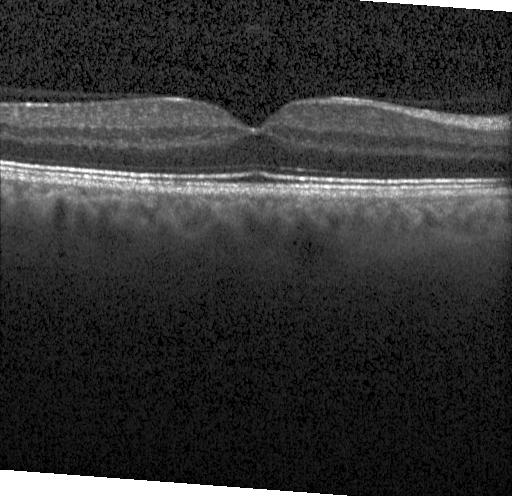

OCT line scan · spectral-domain OCT
This B-scan demonstrates no choroidal neovascularization, no diabetic macular edema, and no drusen.